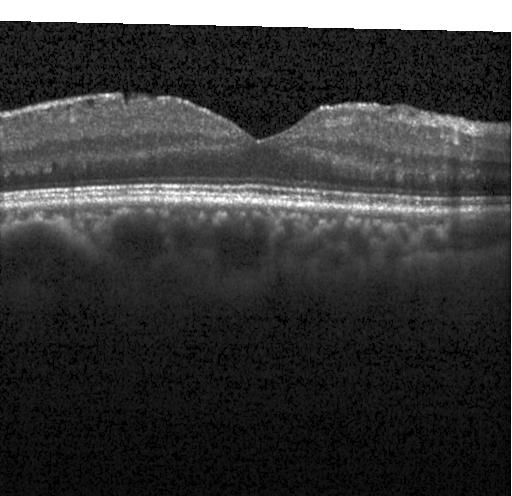

SD-OCT, instrument: Heidelberg Spectralis, OCT B-scan — Diagnosis: no evidence of choroidal neovascularization, diabetic macular edema, or drusen.